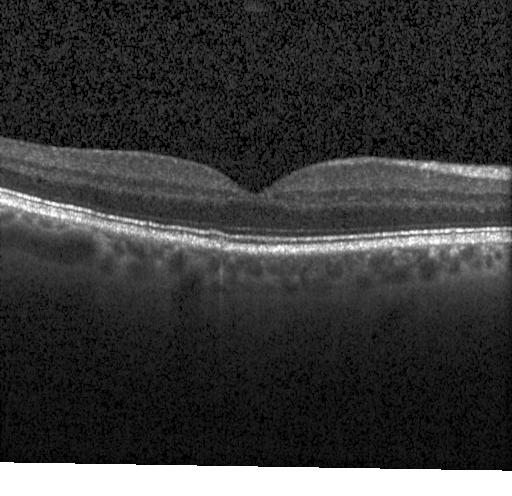

Finding: no choroidal neovascularization, diabetic macular edema, or drusen.